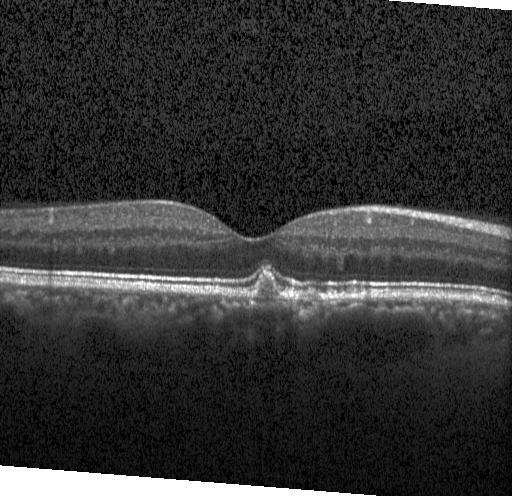

Macular OCT: drusen.